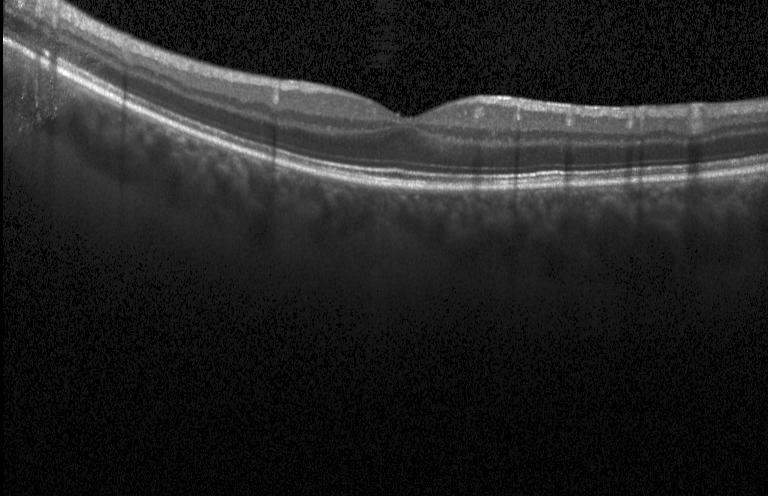
Fovea-centered, retinal OCT cross-section, SD-OCT.
This B-scan demonstrates neither choroidal neovascularization, diabetic macular edema, nor drusen.